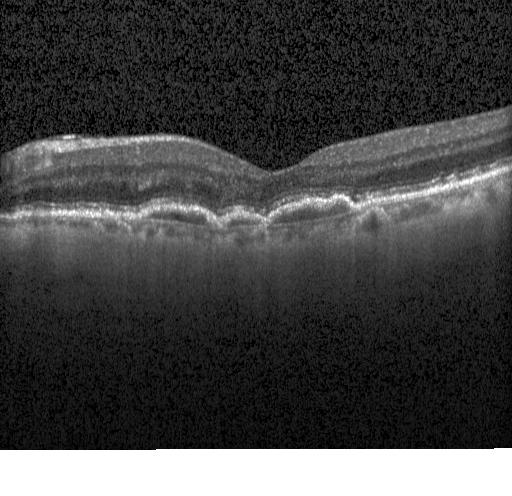

Through the macula. Retinal OCT cross-section. Acquired on a Heidelberg Spectralis.
Diagnosis: a choroidal neovascular membrane.